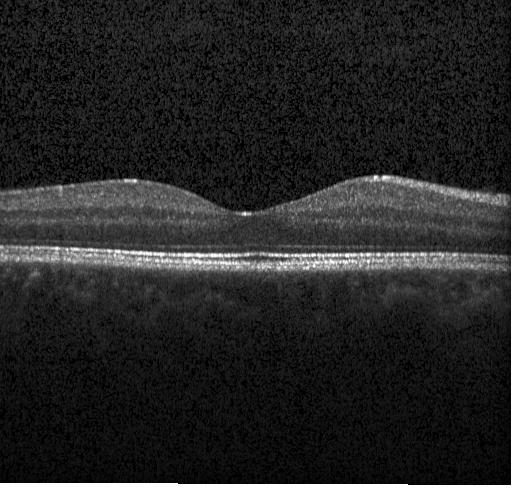

Finding: neither choroidal neovascularization, diabetic macular edema, nor drusen.